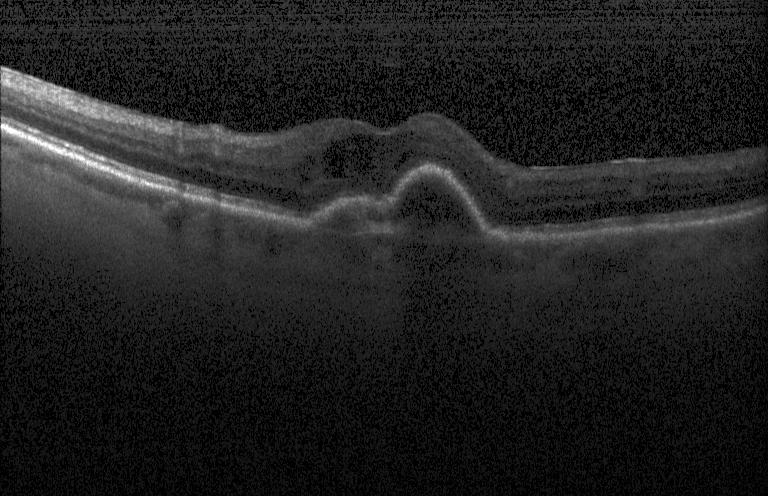 CNV.